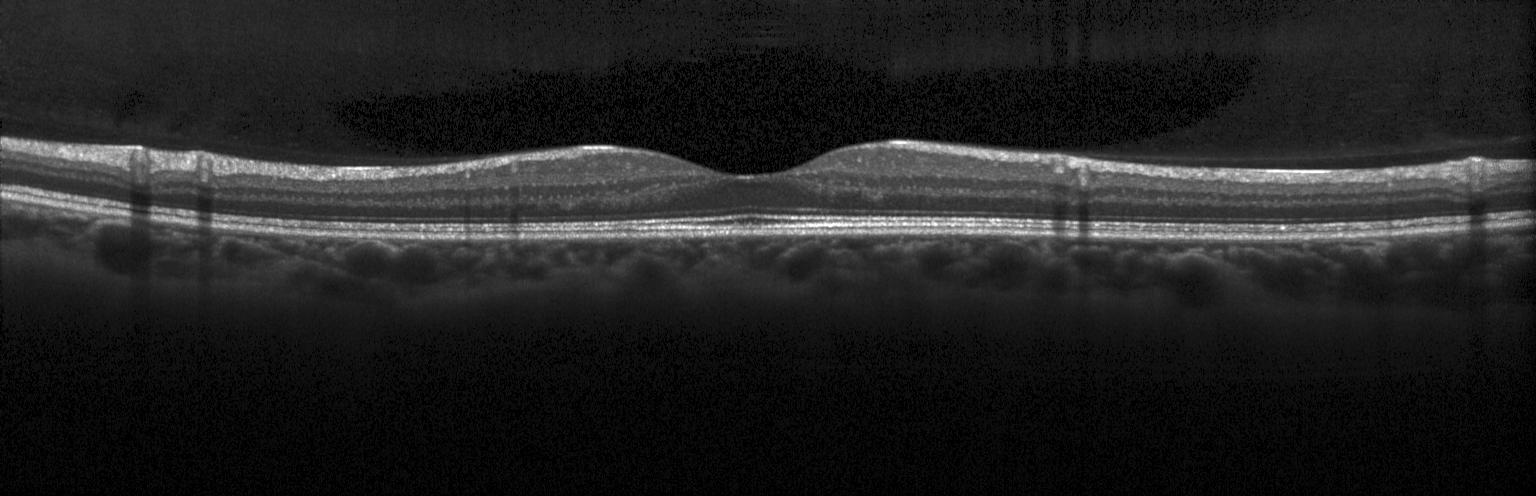 Diagnosis: neither CNV, DME, nor drusen.